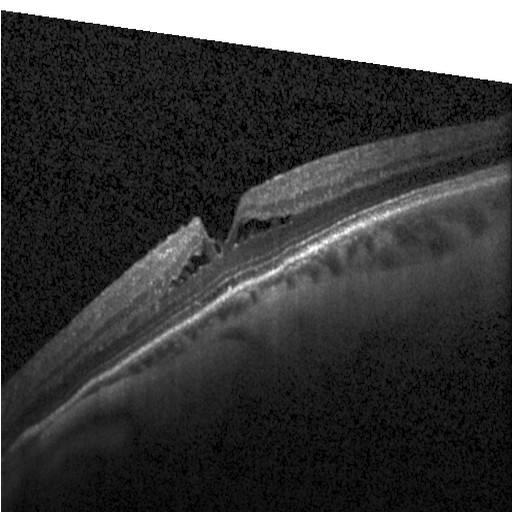

Spectral-domain OCT; Heidelberg Spectralis OCT system; centered on the fovea; retinal OCT cross-section — Assessment: diabetic macular edema (DME).